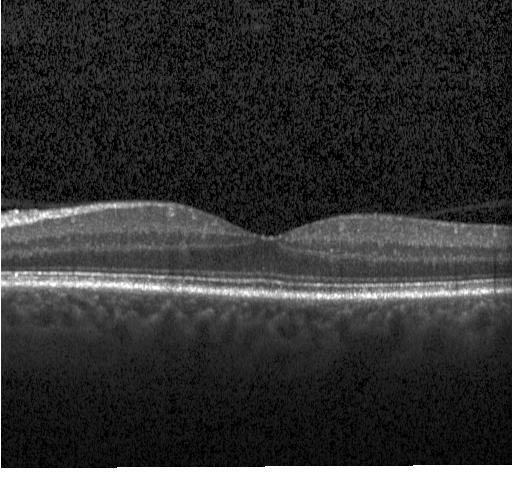 Macular OCT: neither choroidal neovascularization, diabetic macular edema, nor drusen.